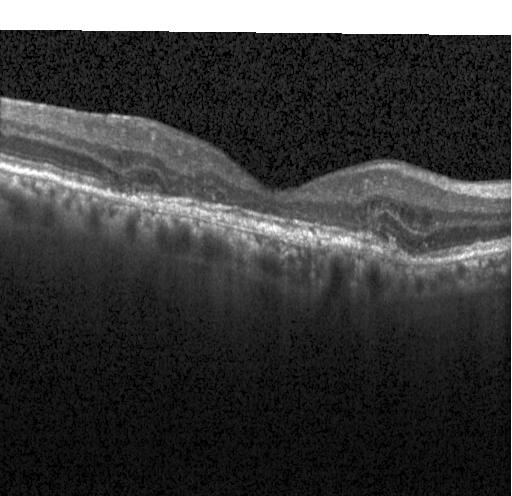

OCT B-scan; acquired on a Heidelberg Spectralis.
A choroidal neovascular membrane.